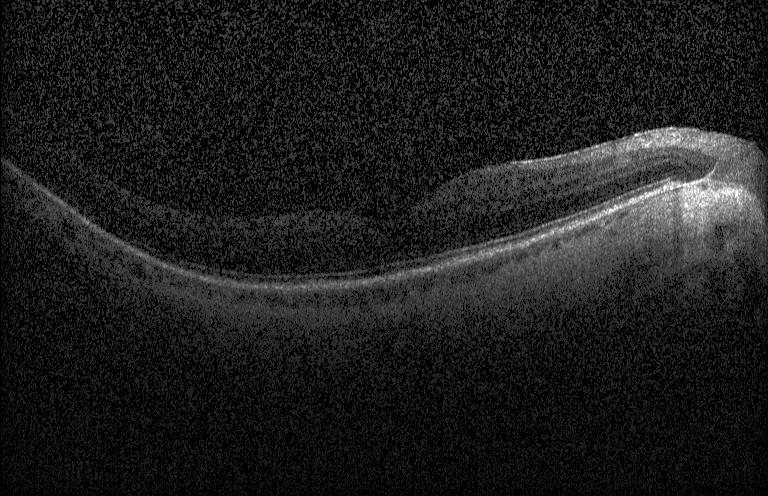

This B-scan demonstrates neither choroidal neovascularization, diabetic macular edema, nor drusen.